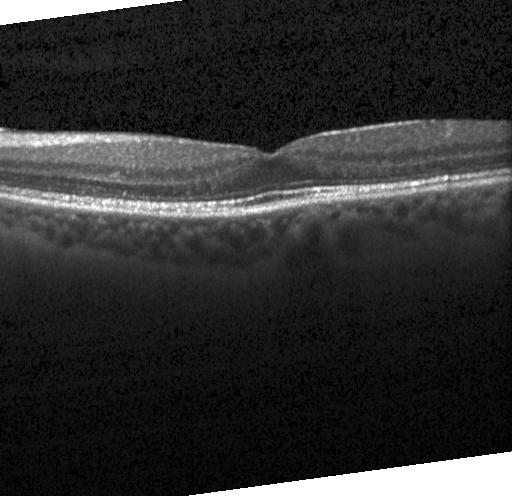

Optical coherence tomography scan. No evidence of choroidal neovascularization, diabetic macular edema, or drusen.